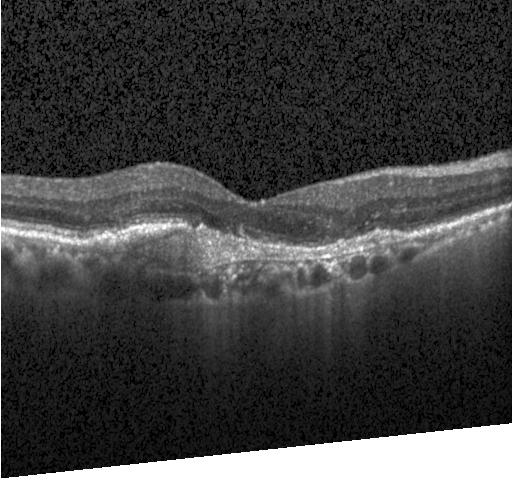 OCT finding: a choroidal neovascular membrane.